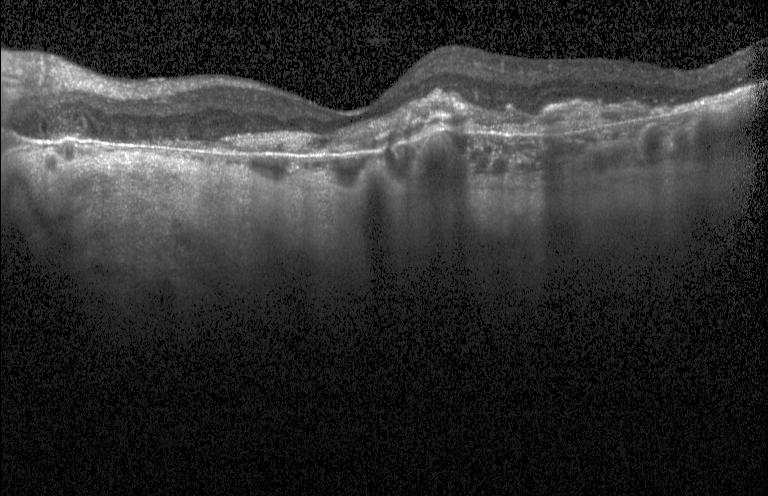
OCT B-scan showing choroidal neovascularization.